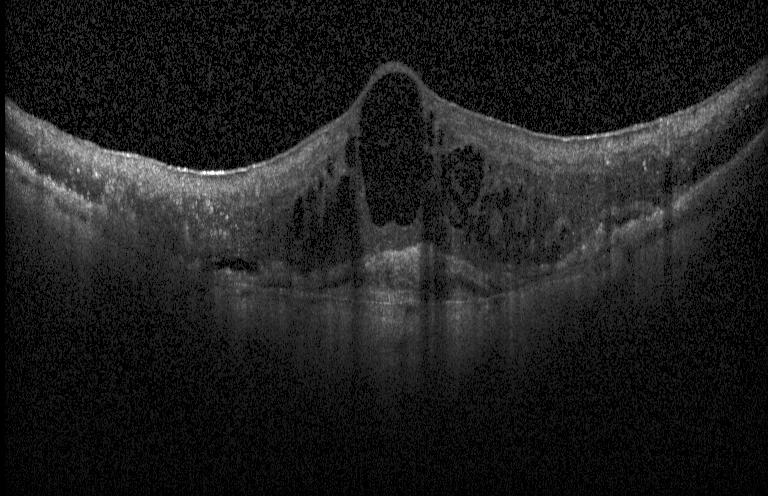 Choroidal neovascularization (CNV).